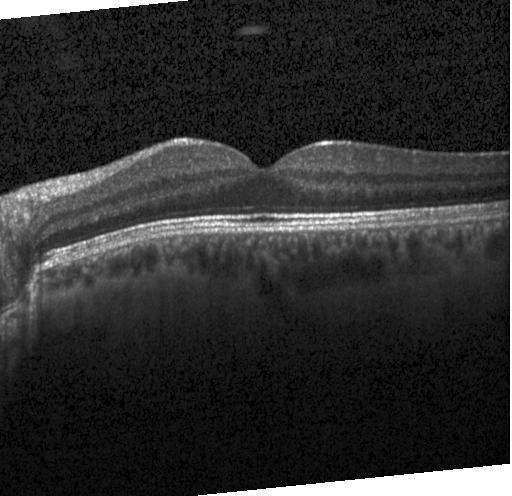
Retinal OCT cross-section showing no choroidal neovascularization, no diabetic macular edema, and no drusen.